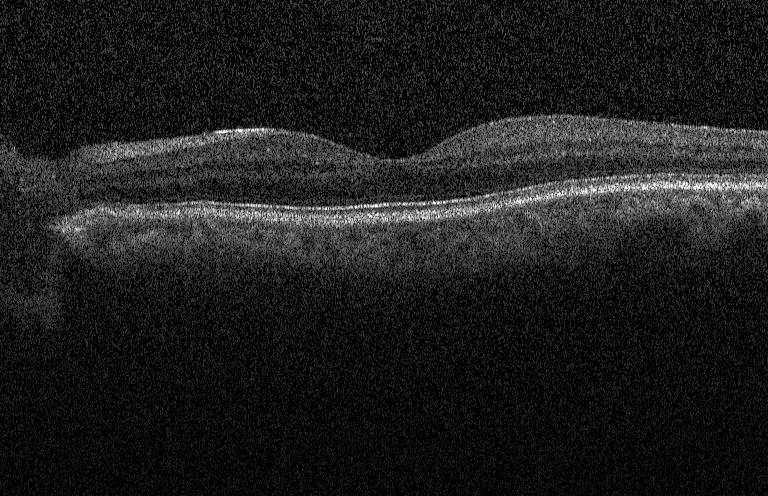

OCT finding: no choroidal neovascularization, diabetic macular edema, or drusen.